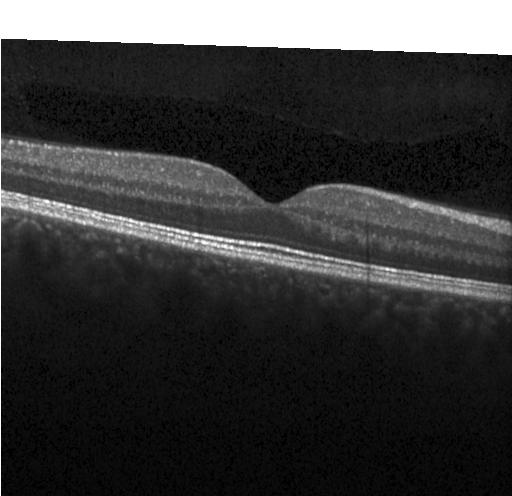

OCT B-scan — OCT finding: no choroidal neovascularization, no diabetic macular edema, and no drusen.